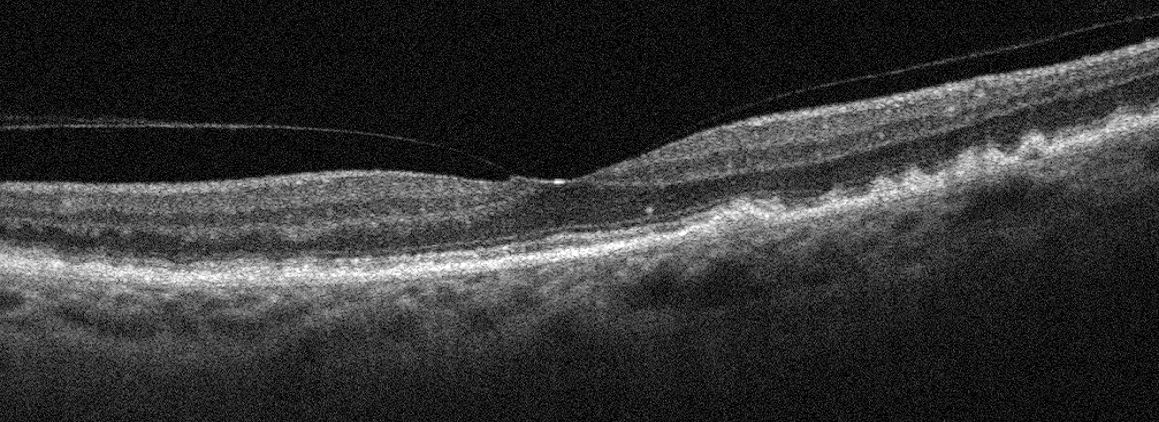 Optical coherence tomography B-scan; fovea-centered; left eye. Dx: AMD.